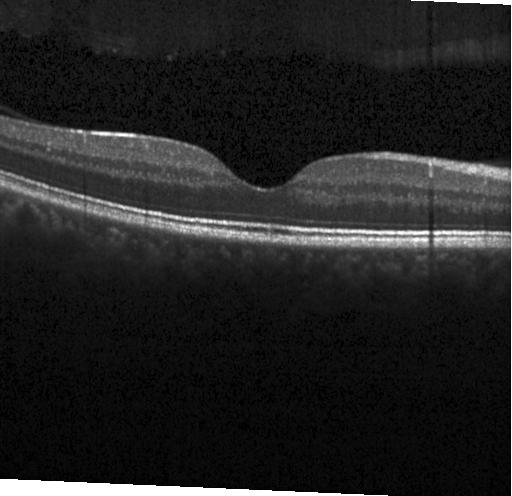 Spectral-domain OCT B-scan: neither choroidal neovascularization, diabetic macular edema, nor drusen.